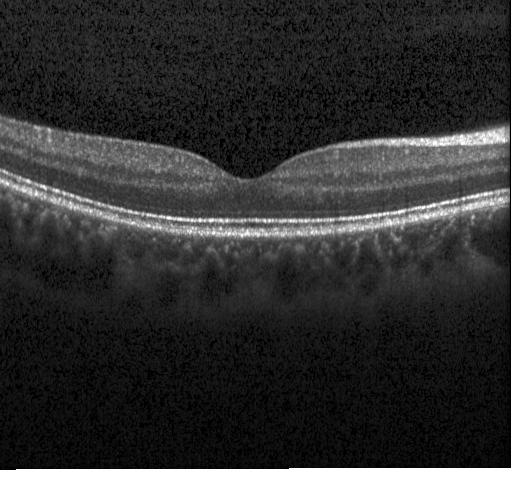

Finding: neither choroidal neovascularization, diabetic macular edema, nor drusen.